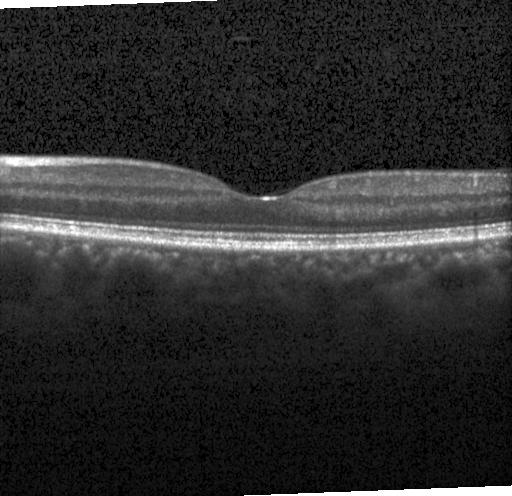

No evidence of choroidal neovascularization, diabetic macular edema, or drusen.